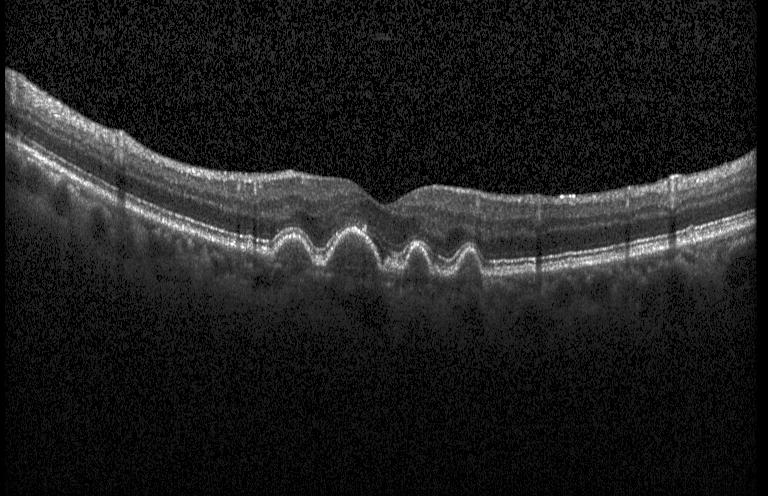 Diagnosis: multiple drusen.